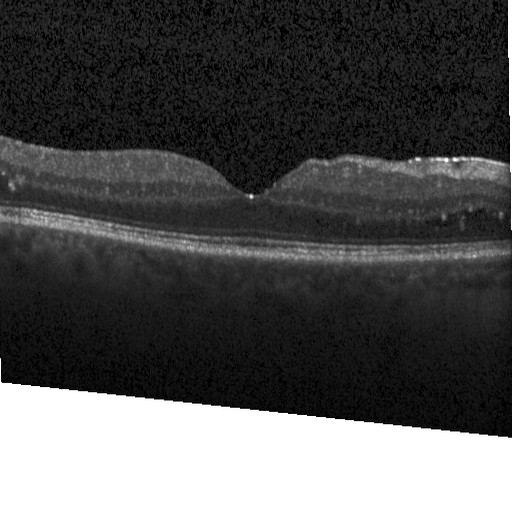
OCT B-scan. Spectral-domain OCT. Instrument: Heidelberg Spectralis. Macular scan.
Impression: DME.